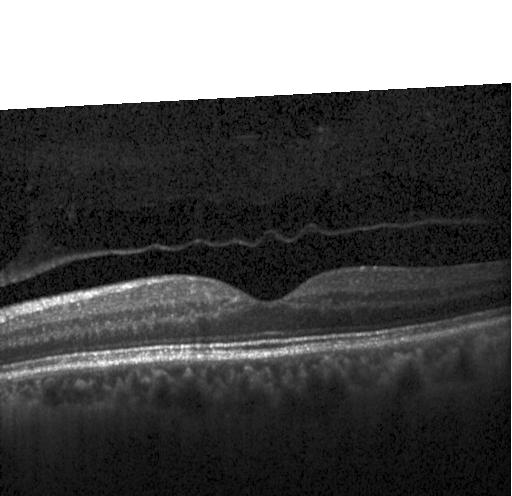
Optical coherence tomography scan · SD-OCT · acquired on a Heidelberg Spectralis — Diagnosis: no choroidal neovascularization, diabetic macular edema, or drusen.